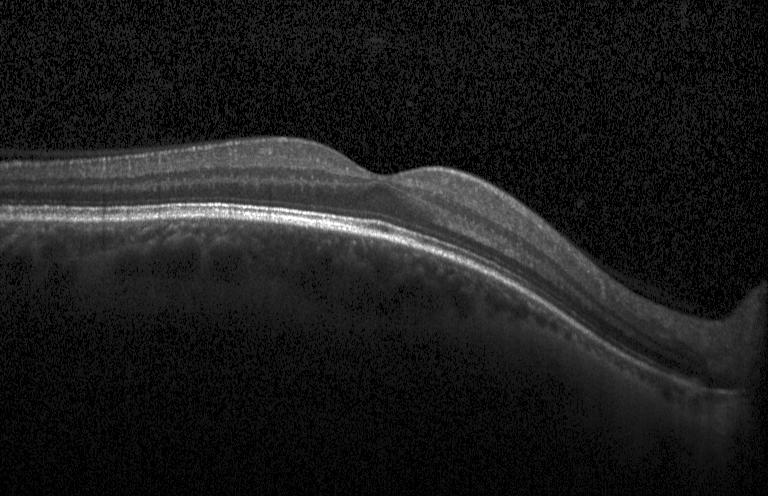 OCT B-scan showing no CNV, DME, or drusen.